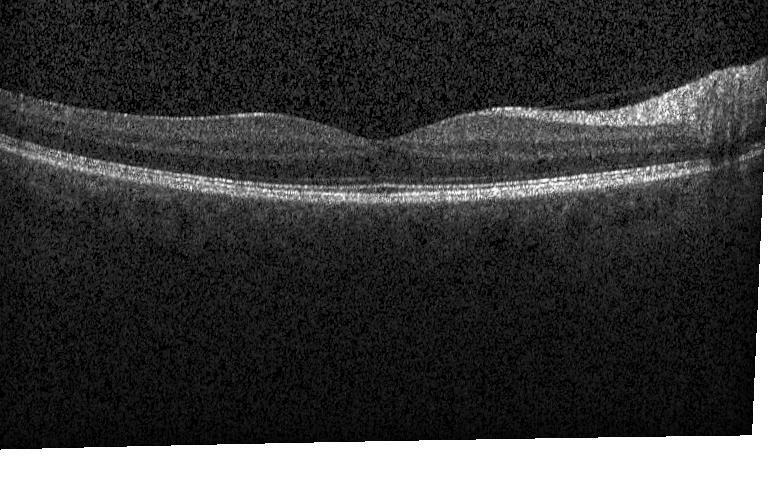

Spectral-domain OCT, retinal OCT B-scan, horizontal scan through the fovea, Heidelberg Spectralis
Diagnosis: no choroidal neovascularization, no diabetic macular edema, and no drusen.